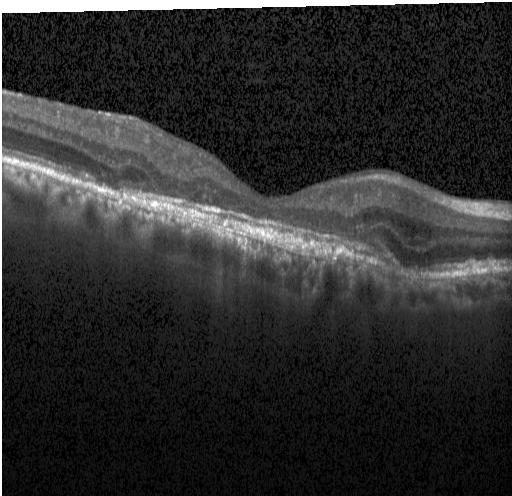 Retinal OCT B-scan, Heidelberg Spectralis OCT system, spectral-domain optical coherence tomography.
Dx: choroidal neovascularization.